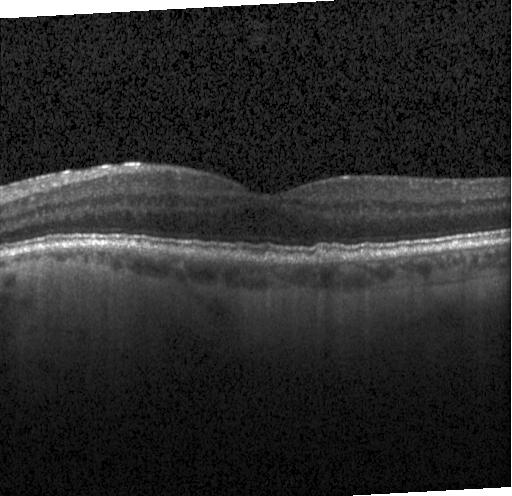
Horizontal scan through the fovea · acquired on a Heidelberg Spectralis · spectral-domain OCT · OCT B-scan — Macular OCT: drusen.